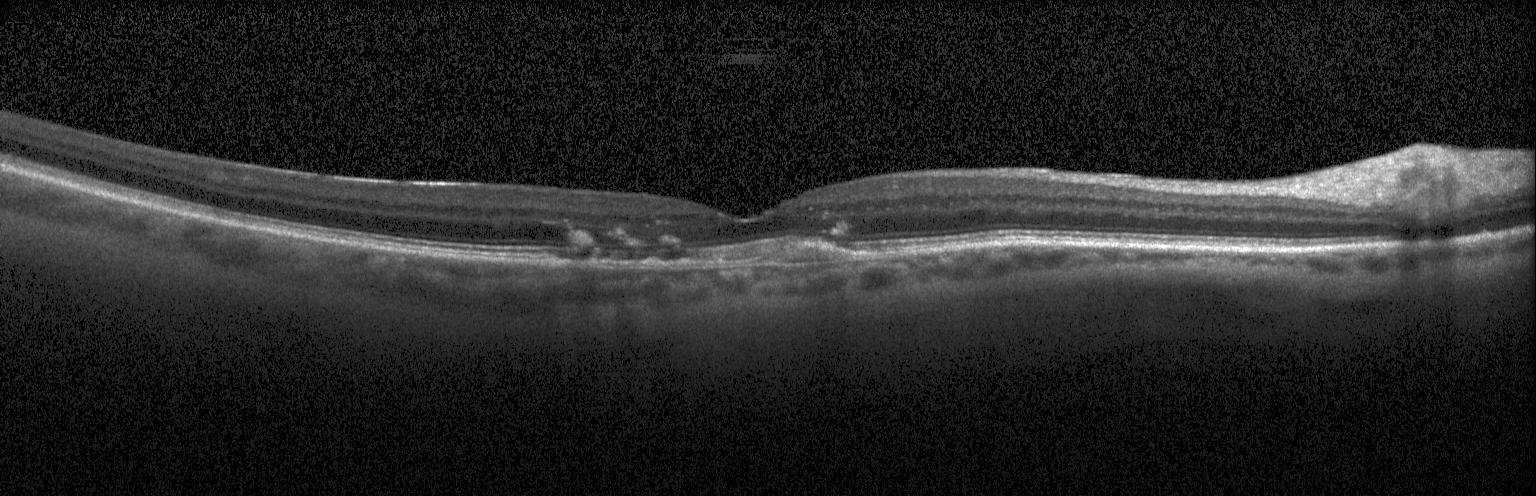
Macular scan. Retinal OCT B-scan. Heidelberg Spectralis OCT system. Spectral-domain OCT — Finding: a choroidal neovascular membrane.